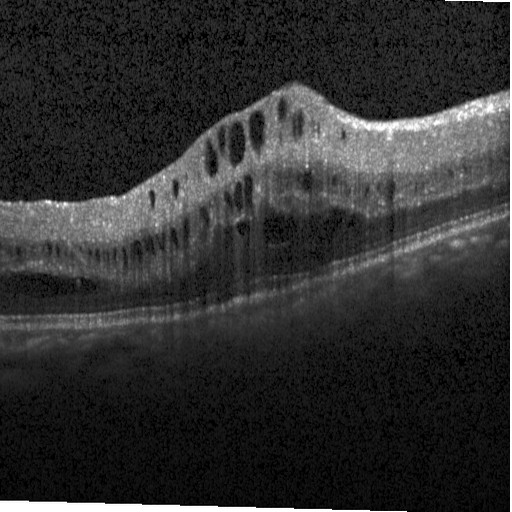 This B-scan demonstrates diabetic macular edema.